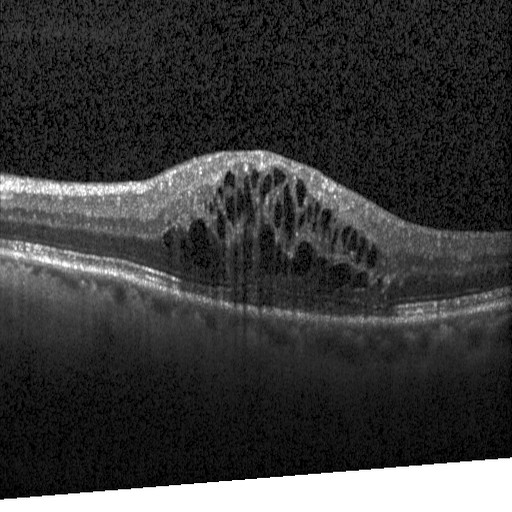

OCT finding: diabetic macular edema (DME).